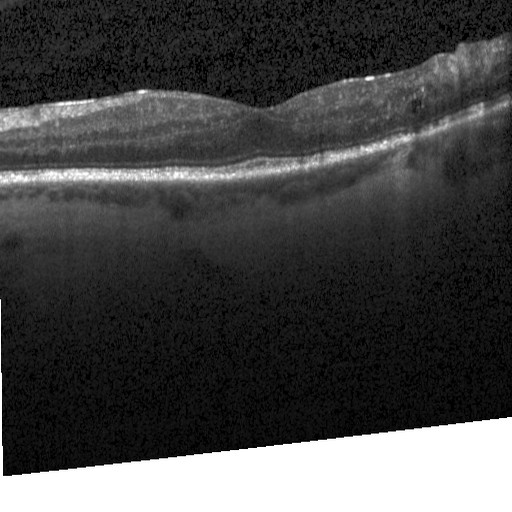

Optical coherence tomography B-scan · fovea-centered · spectral-domain optical coherence tomography · instrument: Heidelberg Spectralis. Diagnosis: DME.